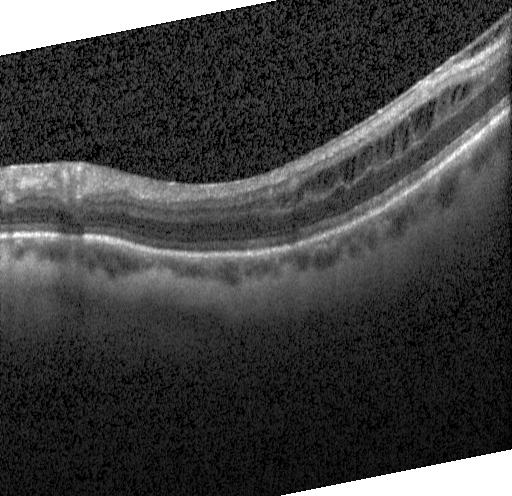

Macular OCT demonstrating DME.